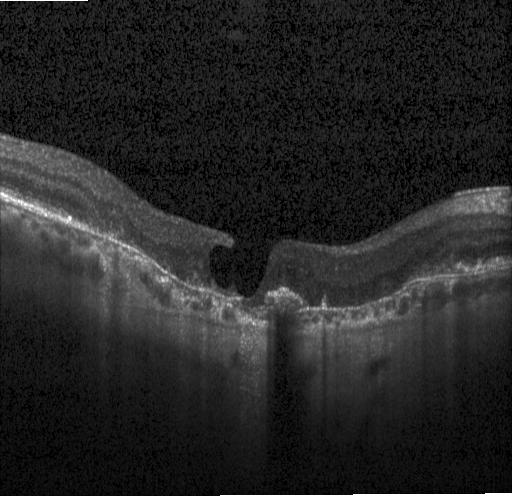

OCT B-scan · spectral-domain optical coherence tomography. OCT finding: a choroidal neovascular membrane.